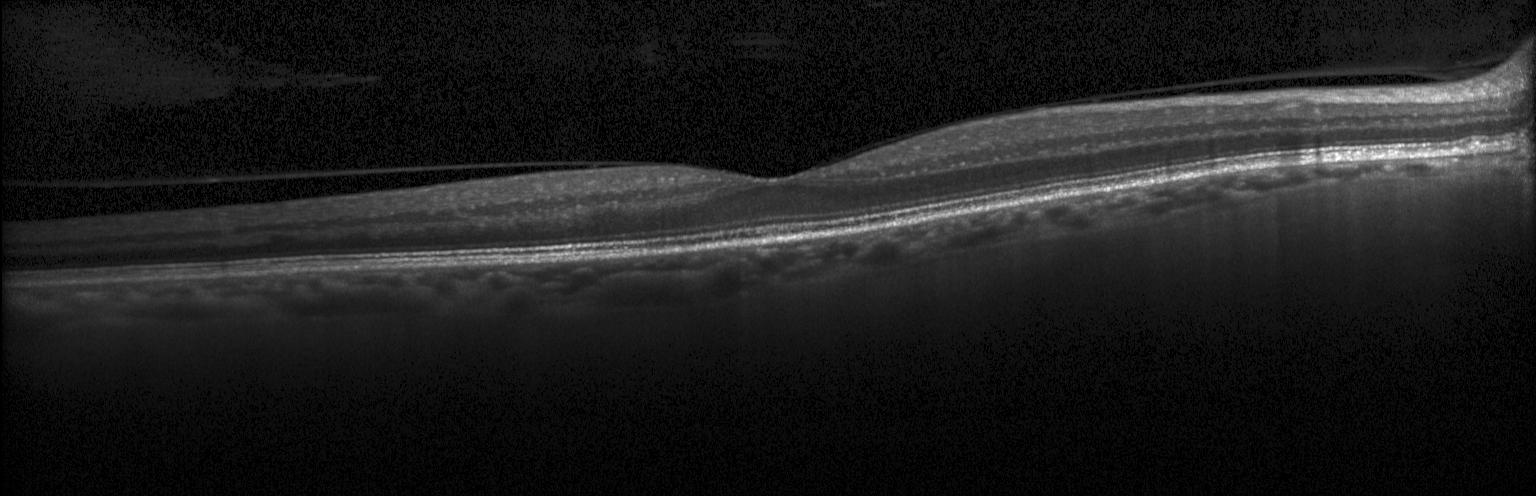

OCT B-scan showing neither CNV, DME, nor drusen.